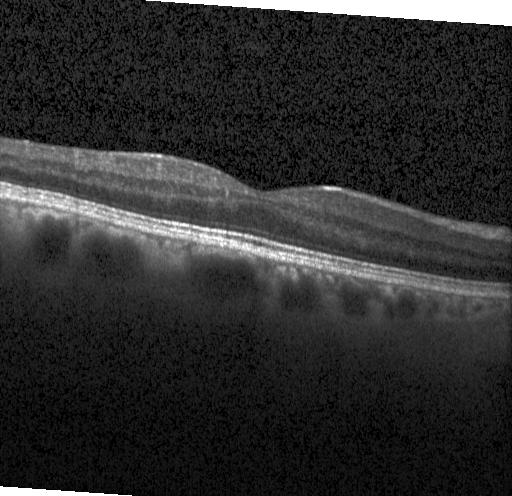

Diagnosis: no CNV, DME, or drusen.